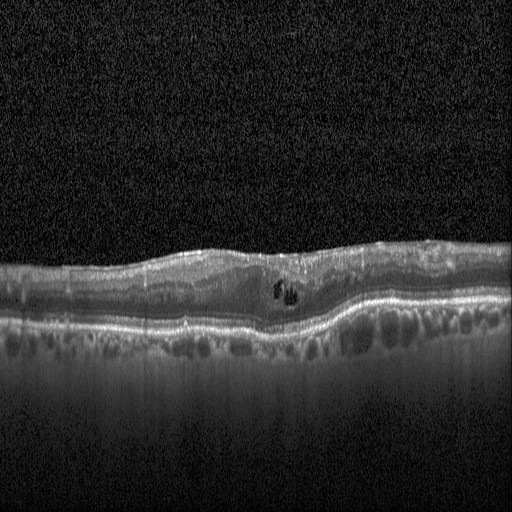 Retinal OCT B-scan.
Diagnosis: diabetic macular edema.